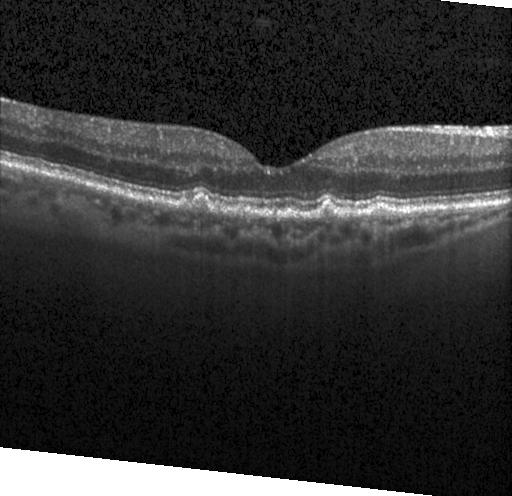

Impression: multiple drusen.